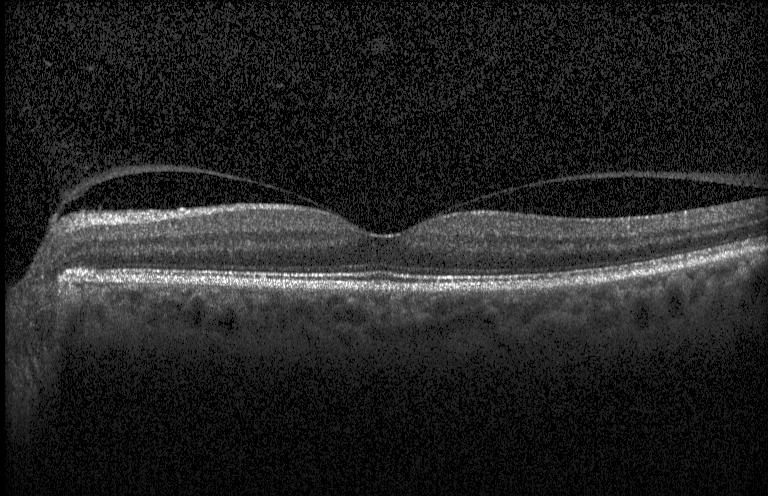

Finding: neither choroidal neovascularization, diabetic macular edema, nor drusen.